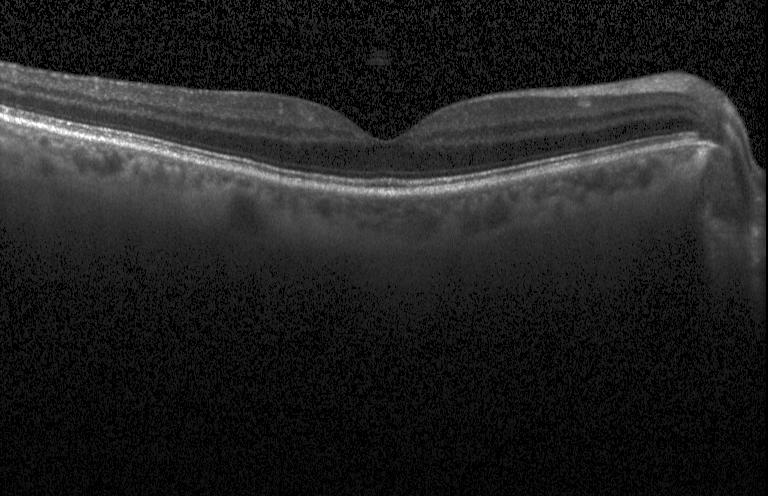

OCT B-scan — Diagnosis: no evidence of choroidal neovascularization, diabetic macular edema, or drusen.